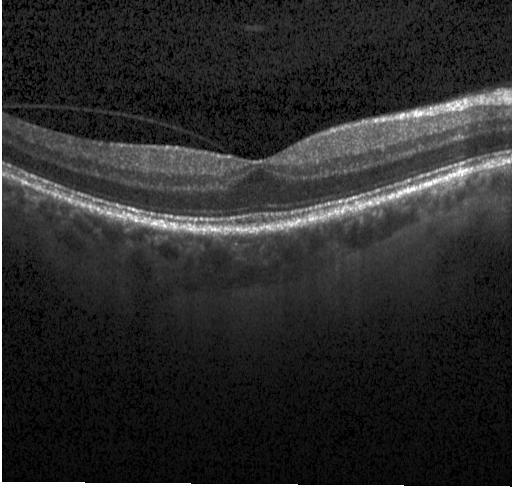 Impression: no choroidal neovascularization, no diabetic macular edema, and no drusen.